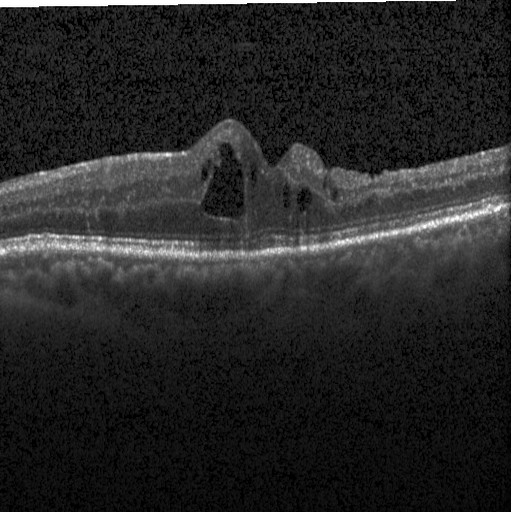 OCT finding: diabetic macular edema (DME).